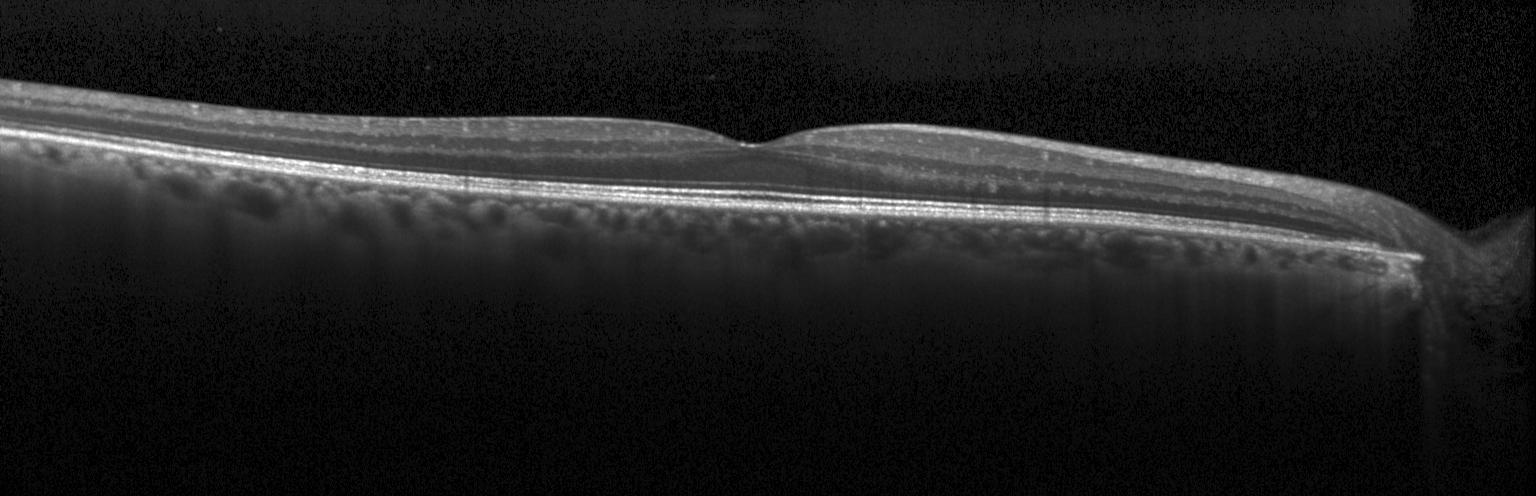
Macular OCT: no CNV, no DME, and no drusen.